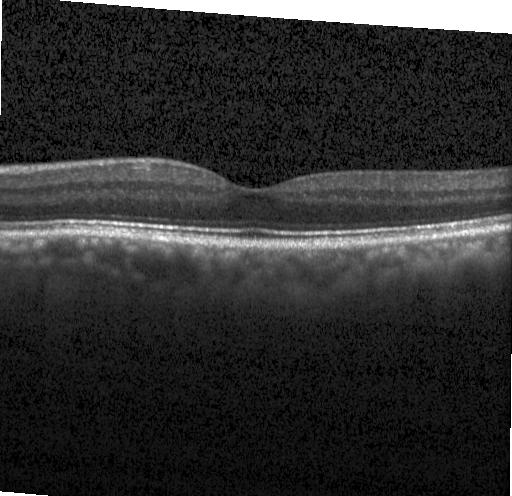

Instrument: Heidelberg Spectralis; retinal OCT B-scan; SD-OCT. Impression: no choroidal neovascularization, no diabetic macular edema, and no drusen.